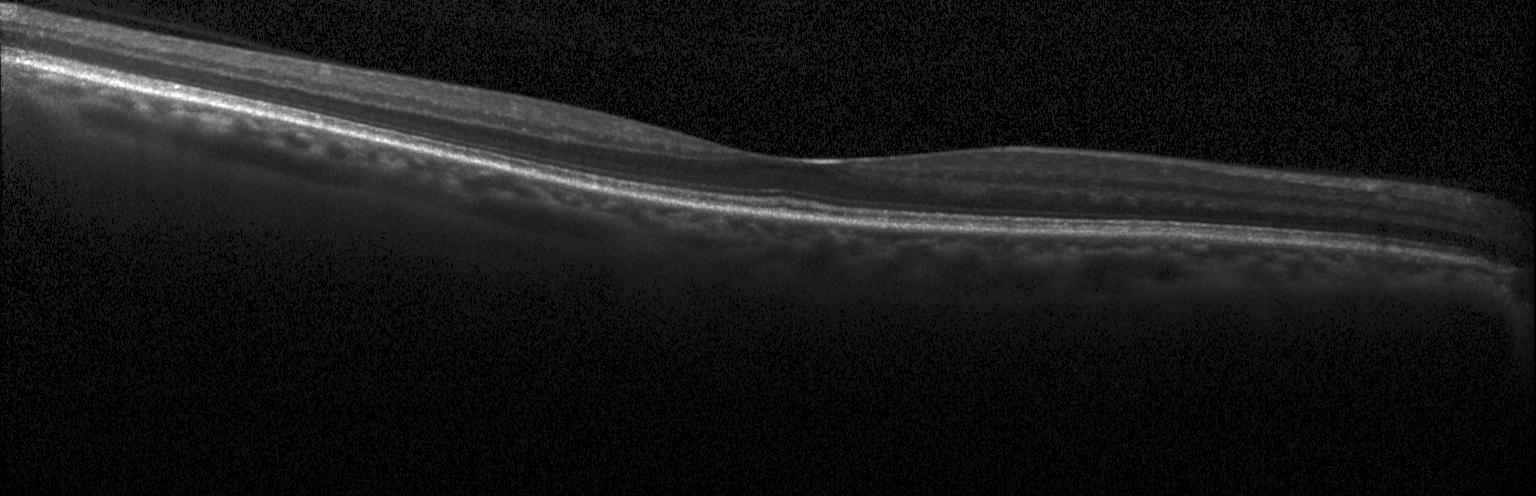

Retinal OCT cross-section. SD-OCT. Heidelberg Spectralis. Diagnosis: no evidence of CNV, DME, or drusen.